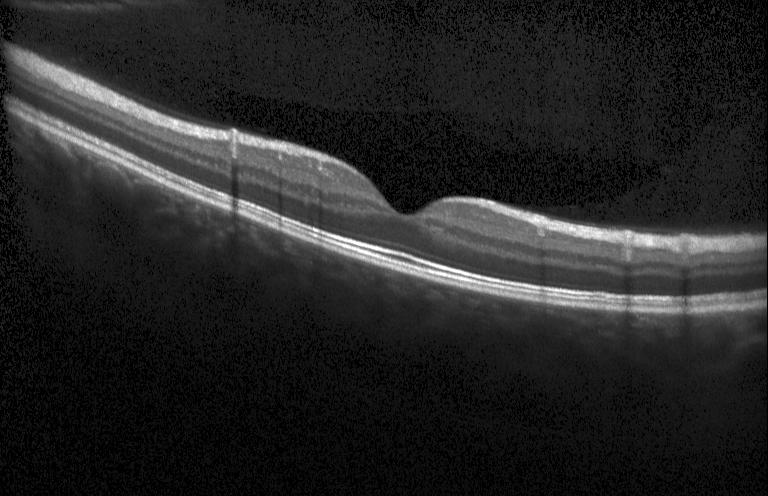

Impression: no choroidal neovascularization, no diabetic macular edema, and no drusen.